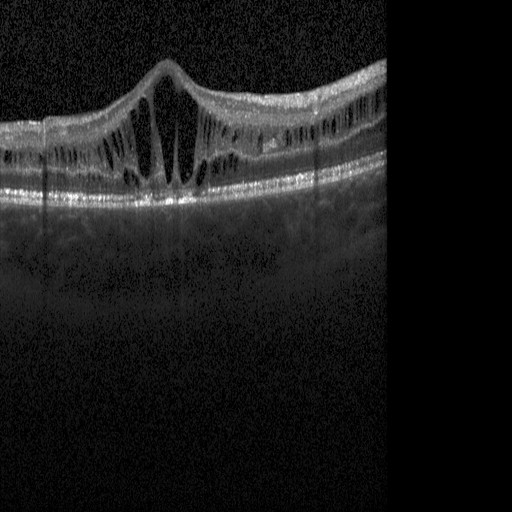 Spectral-domain optical coherence tomography, OCT line scan.
Impression: diabetic macular edema (DME).